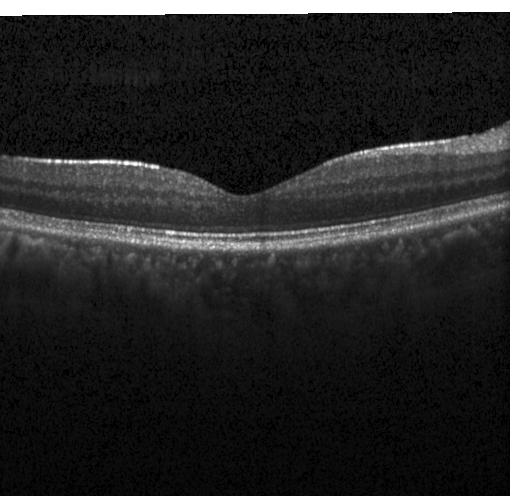

Optical coherence tomography scan · Heidelberg Spectralis · centered on the fovea
Neither choroidal neovascularization, diabetic macular edema, nor drusen.